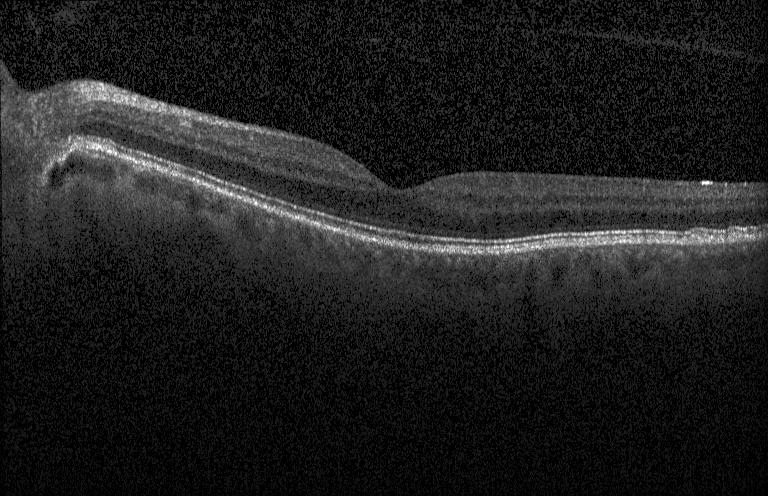 Retinal OCT B-scan; SD-OCT
Finding: neither choroidal neovascularization, diabetic macular edema, nor drusen.